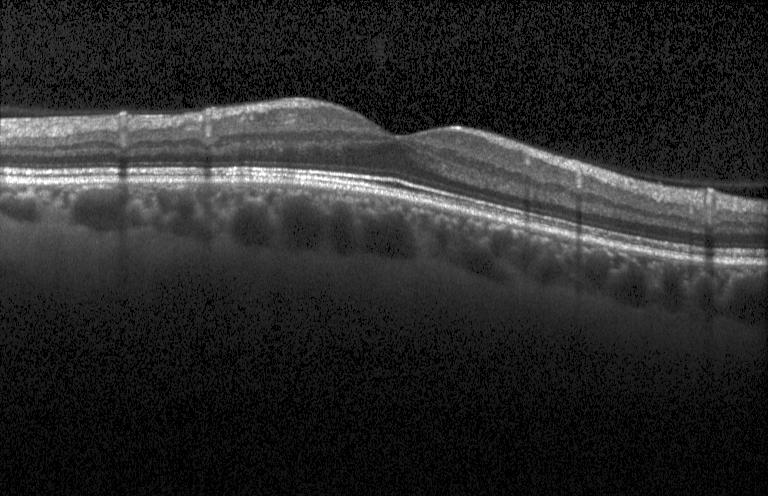

Optical coherence tomography scan · horizontal scan through the fovea · SD-OCT · acquired on a Heidelberg Spectralis.
The scan shows no CNV, no DME, and no drusen.